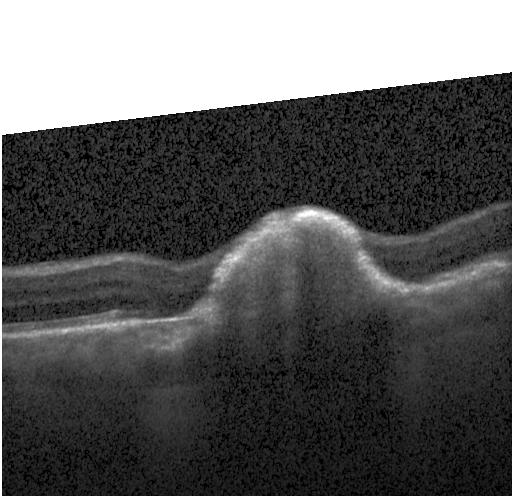

This B-scan demonstrates choroidal neovascularization.